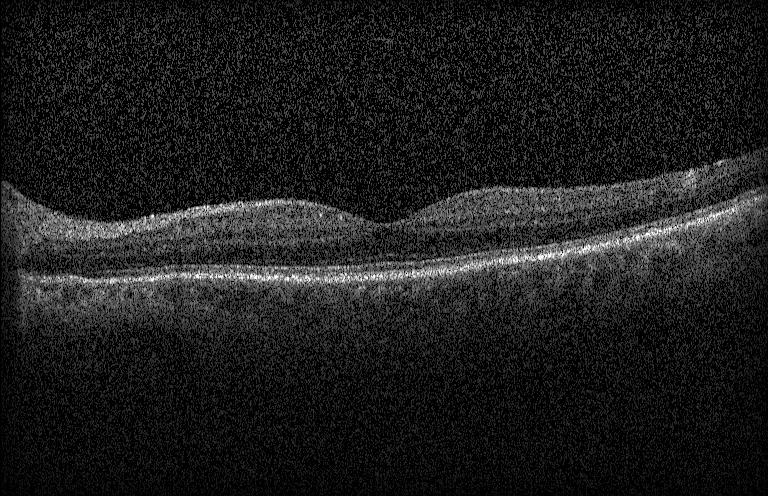

Instrument: Heidelberg Spectralis. Retinal OCT cross-section.
Impression: no CNV, DME, or drusen.